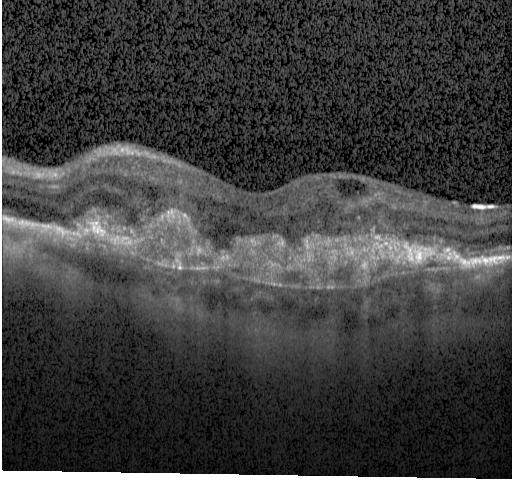

Horizontal scan through the fovea · spectral-domain optical coherence tomography · retinal OCT B-scan — Impression: choroidal neovascularization.